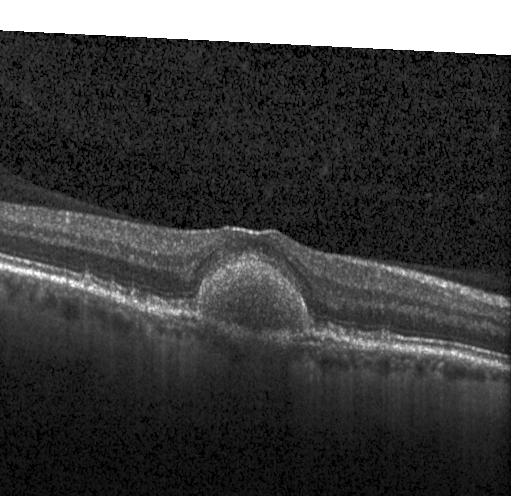 Diagnosis: a choroidal neovascular membrane.